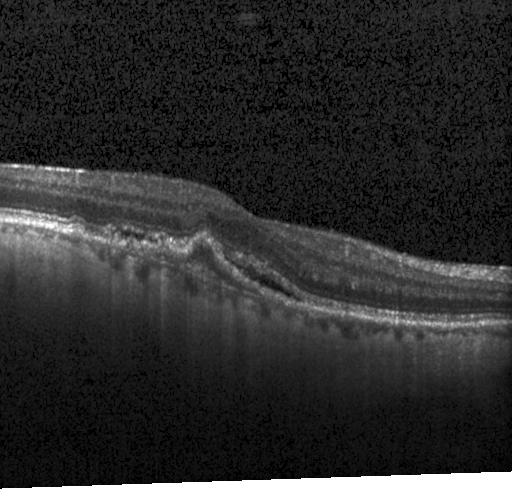 The scan shows choroidal neovascularization (CNV).